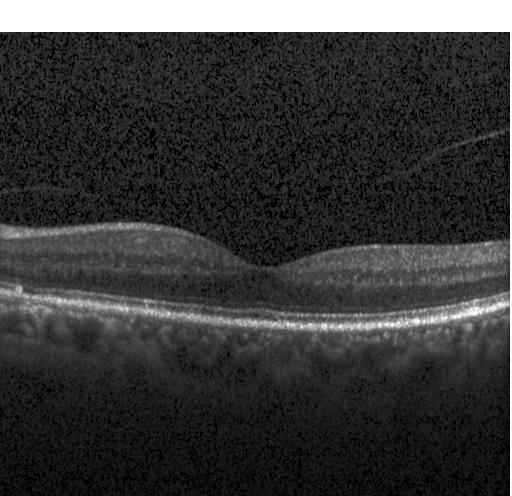

Horizontal scan through the fovea; SD-OCT; acquired on a Heidelberg Spectralis; retinal OCT cross-section. OCT finding: no choroidal neovascularization, diabetic macular edema, or drusen.